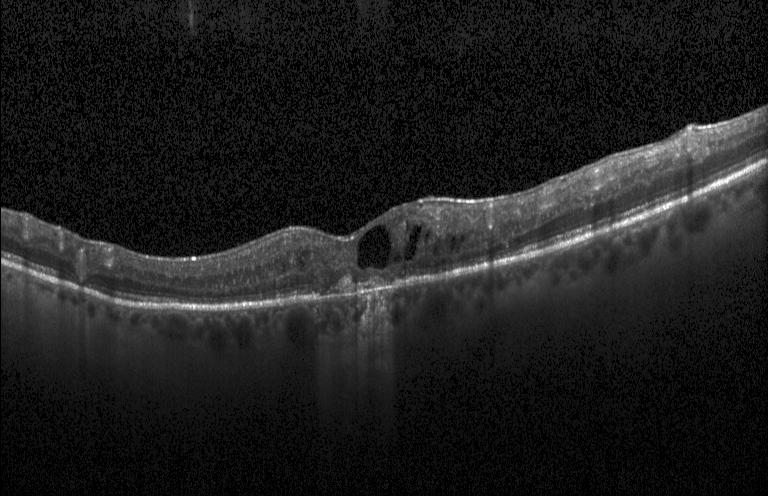 OCT B-scan — Diagnosis: a choroidal neovascular membrane.